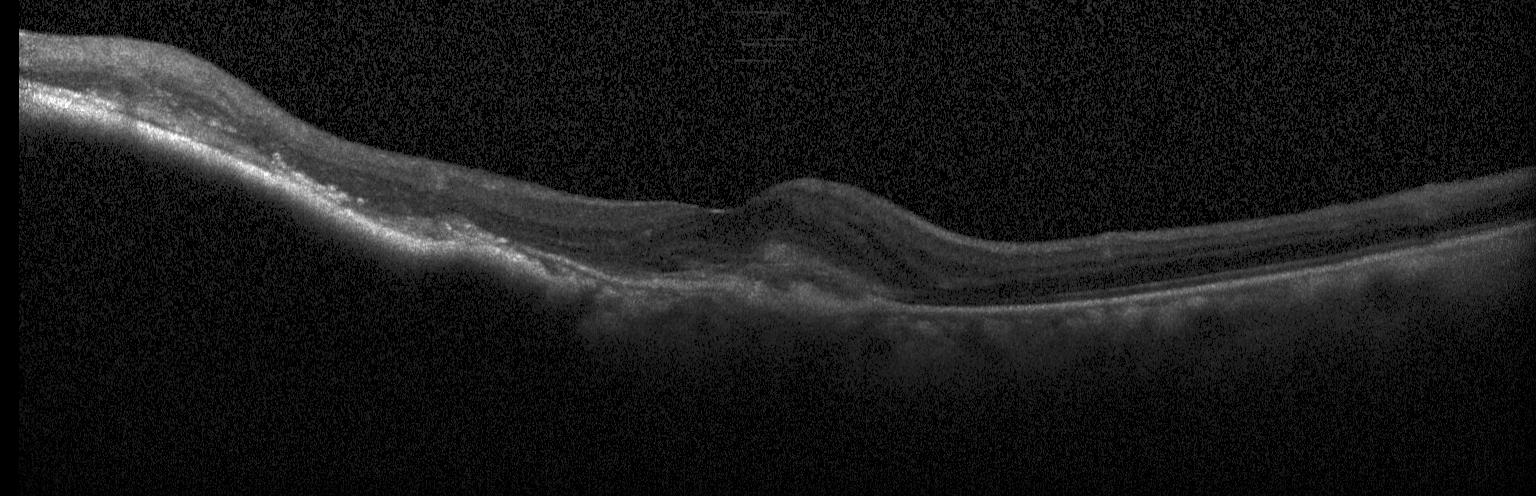
OCT finding: choroidal neovascularization (CNV).